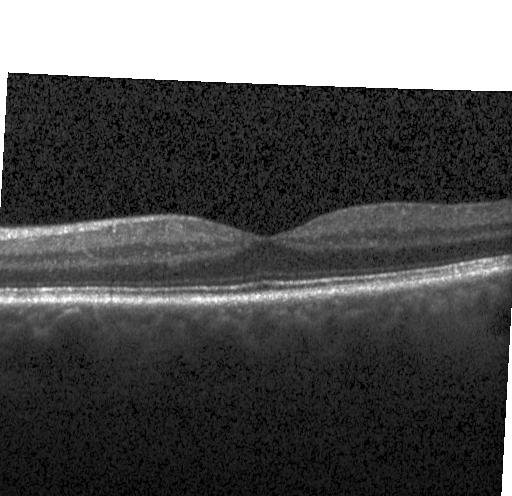

Spectral-domain optical coherence tomography · optical coherence tomography B-scan · centered on the fovea.
Diagnosis: neither choroidal neovascularization, diabetic macular edema, nor drusen.